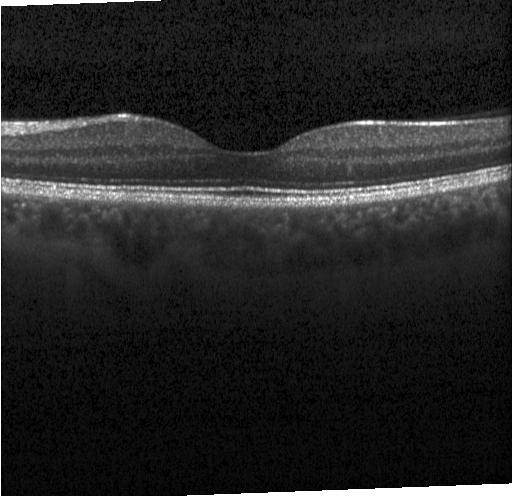 Heidelberg Spectralis, centered on the fovea, OCT B-scan, spectral-domain OCT — Finding: no evidence of choroidal neovascularization, diabetic macular edema, or drusen.